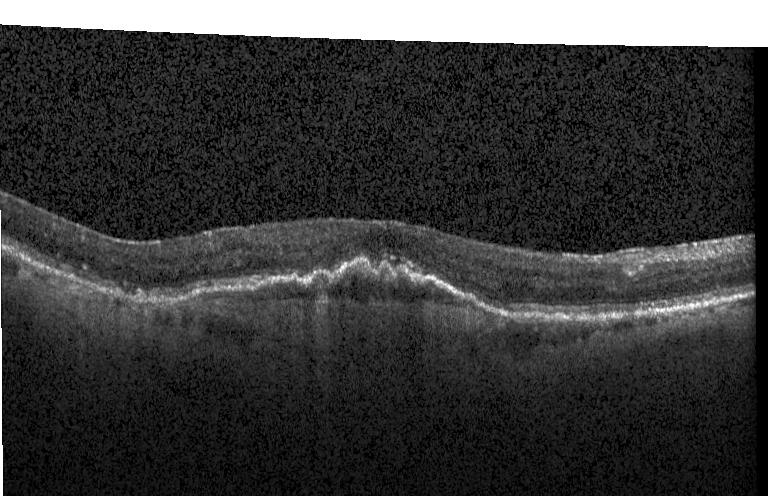 Optical coherence tomography scan — Dx: a choroidal neovascular membrane.